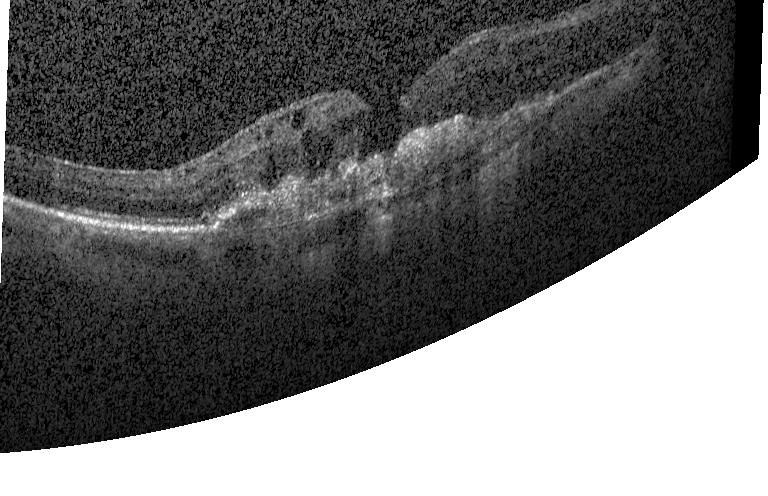 Macular OCT: a choroidal neovascular membrane.